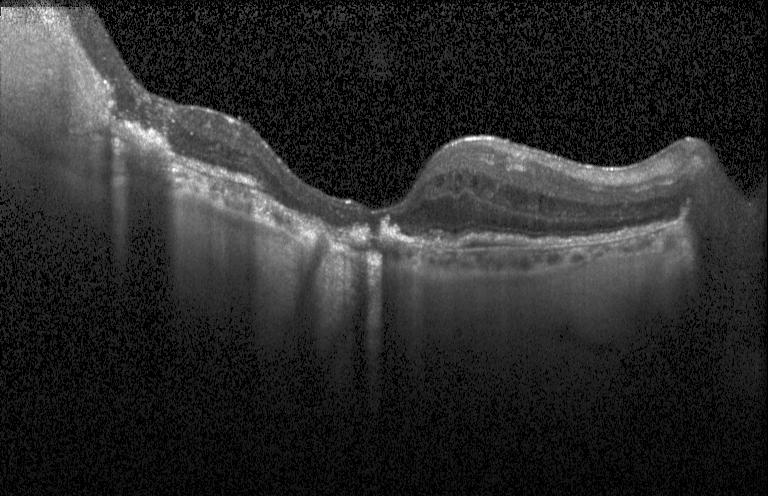 Horizontal scan through the fovea · Heidelberg Spectralis OCT system · optical coherence tomography B-scan · spectral-domain OCT.
Dx: a choroidal neovascular membrane.